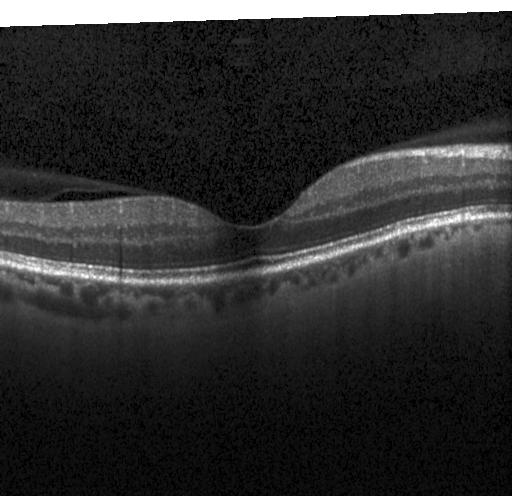
Diagnosis: no choroidal neovascularization, diabetic macular edema, or drusen.